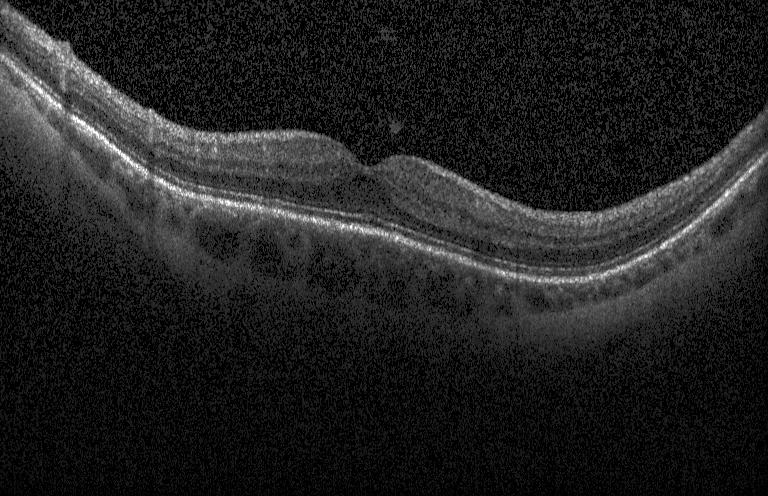 OCT line scan.
Assessment: no choroidal neovascularization, diabetic macular edema, or drusen.